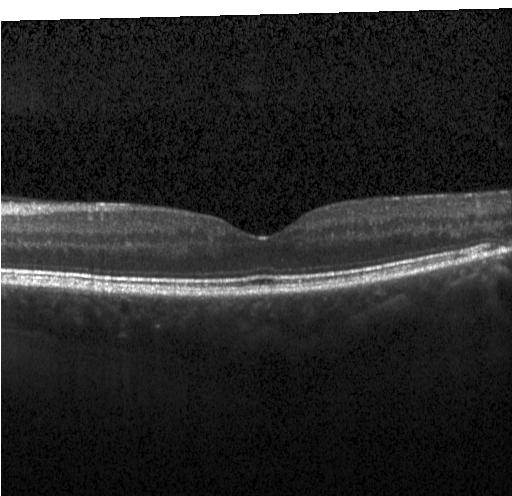
SD-OCT, retinal OCT B-scan, Heidelberg Spectralis OCT system, centered on the fovea. The scan shows no CNV, no DME, and no drusen.